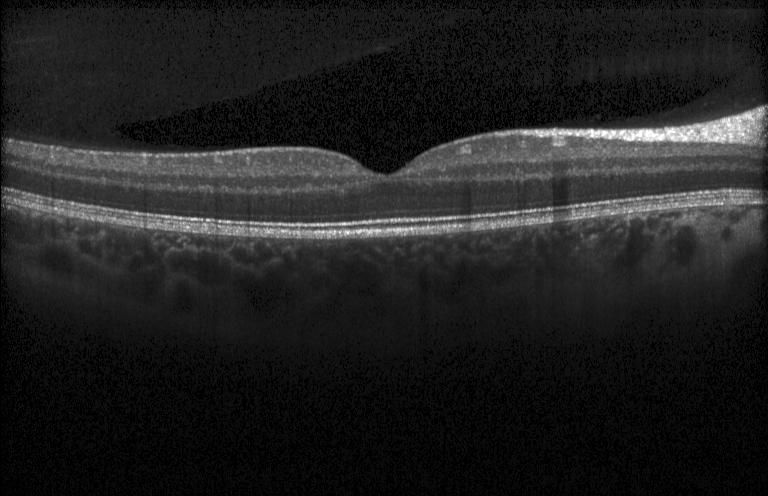

Macular scan. Retinal OCT B-scan — The scan shows neither choroidal neovascularization, diabetic macular edema, nor drusen.